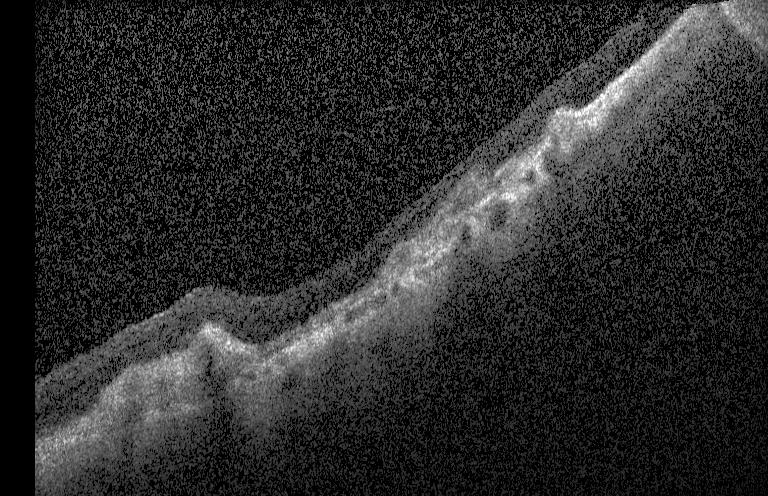

Impression: CNV.